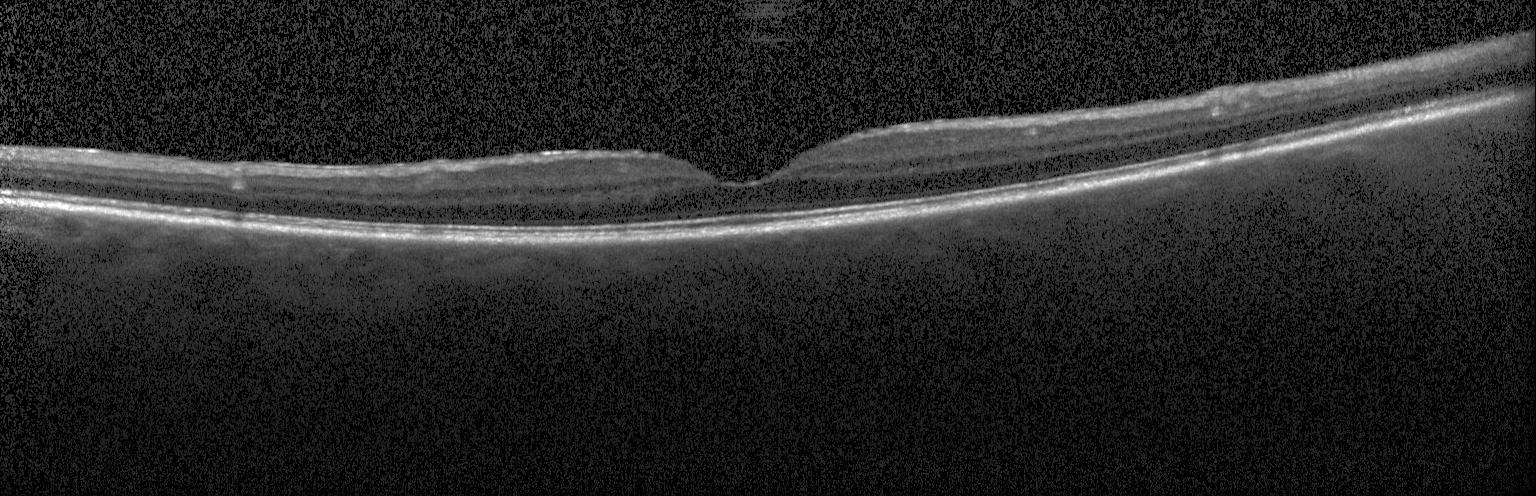 OCT line scan. Heidelberg Spectralis OCT system. Horizontal scan through the fovea — This B-scan demonstrates no CNV, no DME, and no drusen.